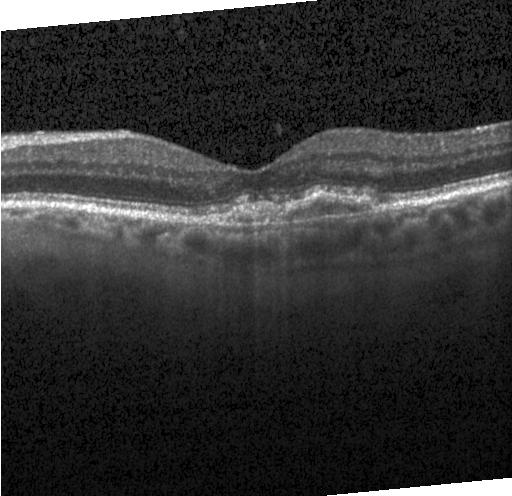
OCT finding: choroidal neovascularization (CNV).